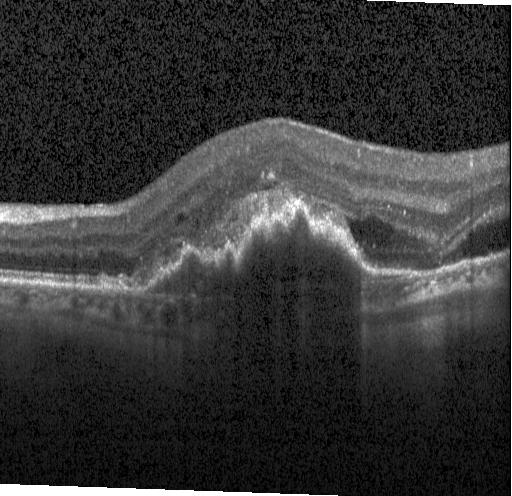
OCT B-scan; SD-OCT; fovea-centered. This B-scan demonstrates a choroidal neovascular membrane.